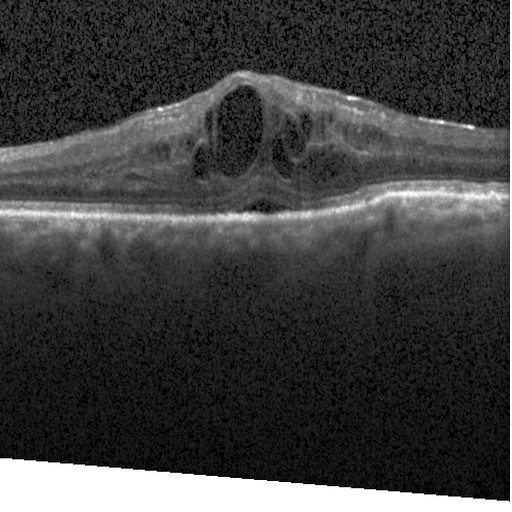 Finding: DME.